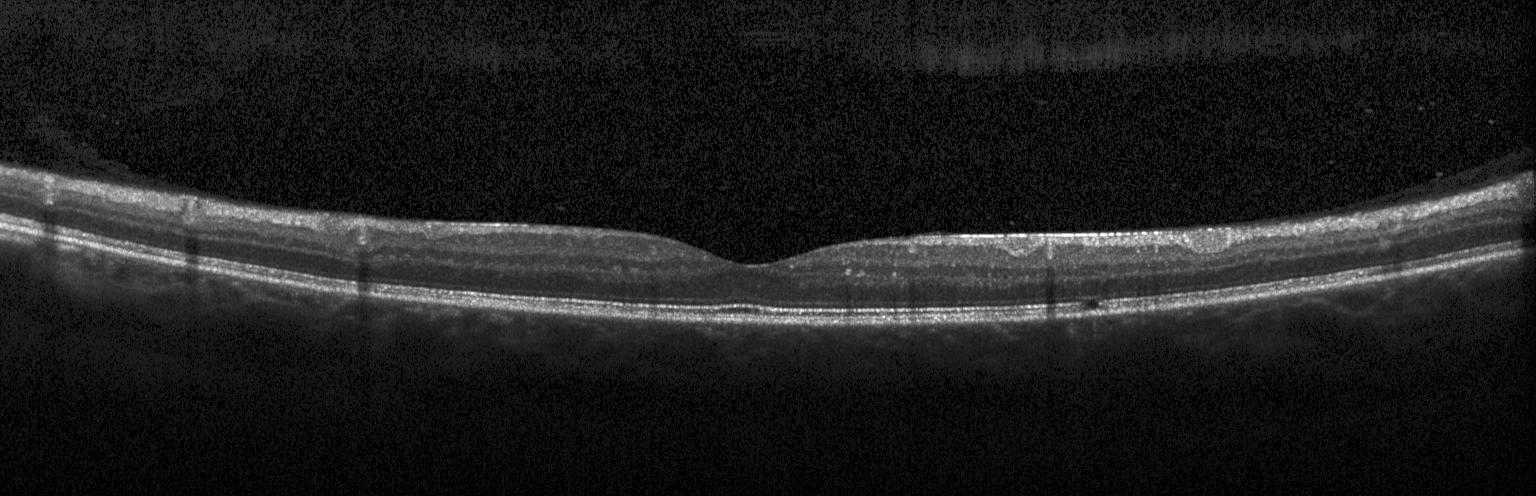 Centered on the fovea · OCT B-scan · acquired on a Heidelberg Spectralis · spectral-domain optical coherence tomography.
Diagnosis: no choroidal neovascularization, no diabetic macular edema, and no drusen.